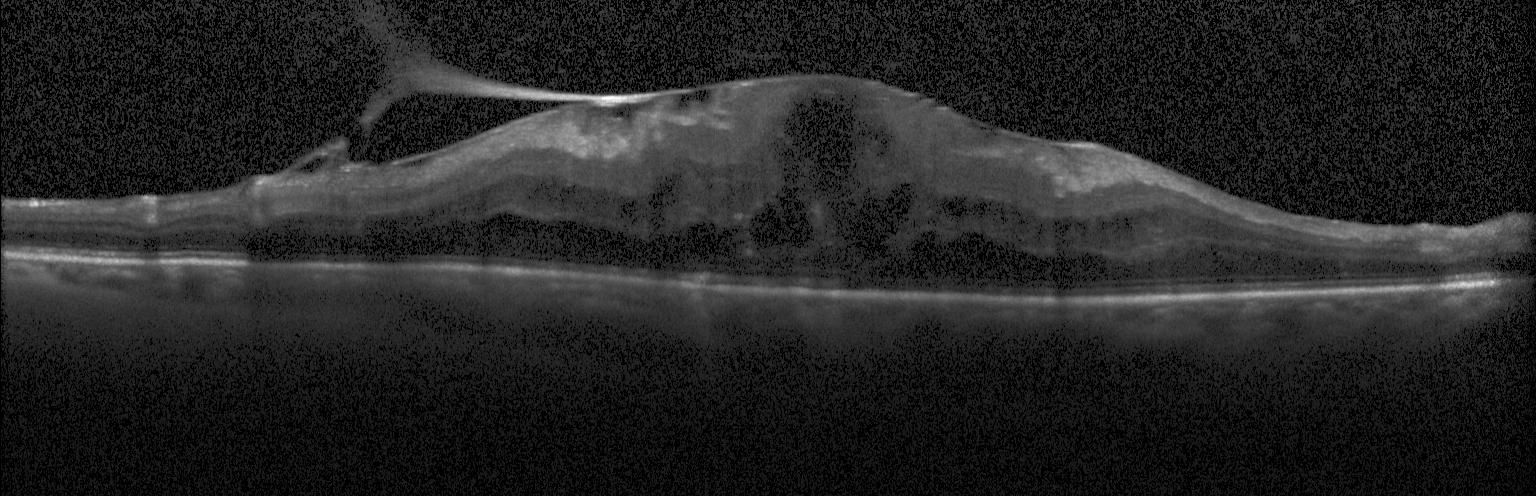
Heidelberg Spectralis OCT system; retinal OCT B-scan.
Finding: diabetic macular edema.